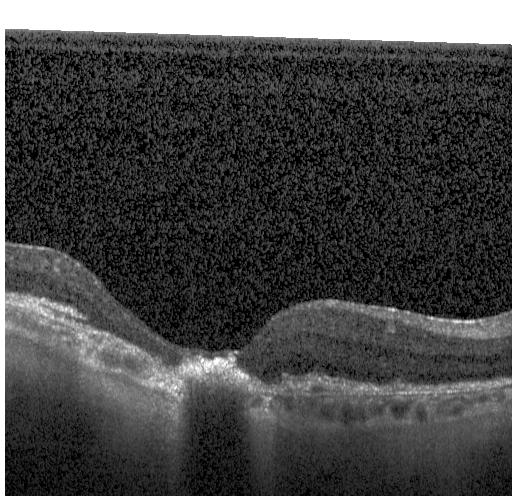 Optical coherence tomography B-scan · horizontal scan through the fovea
Macular OCT: a choroidal neovascular membrane.